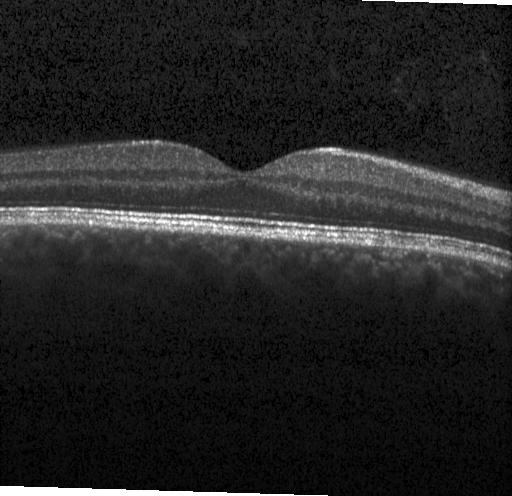
OCT line scan; spectral-domain OCT; horizontal scan through the fovea; instrument: Heidelberg Spectralis.
Finding: no CNV, no DME, and no drusen.